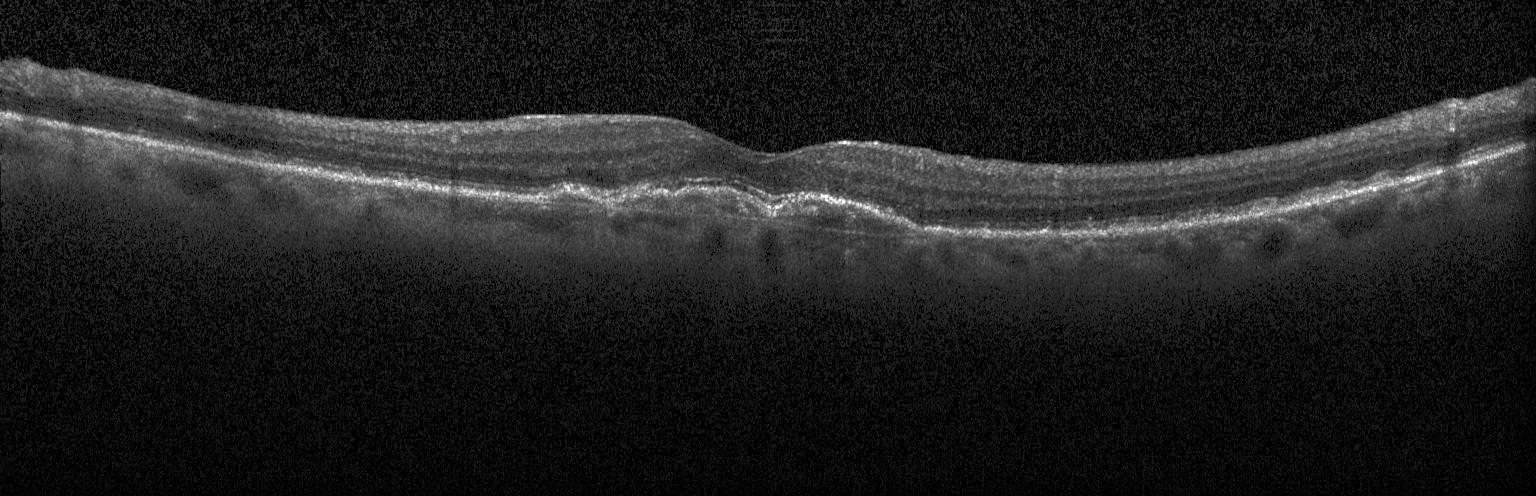 Retinal OCT cross-section.
Finding: CNV.